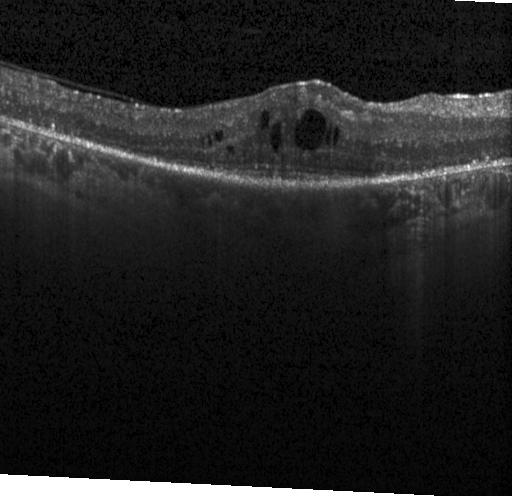
OCT line scan · spectral-domain OCT · acquired on a Heidelberg Spectralis. Macular OCT: diabetic macular edema (DME).